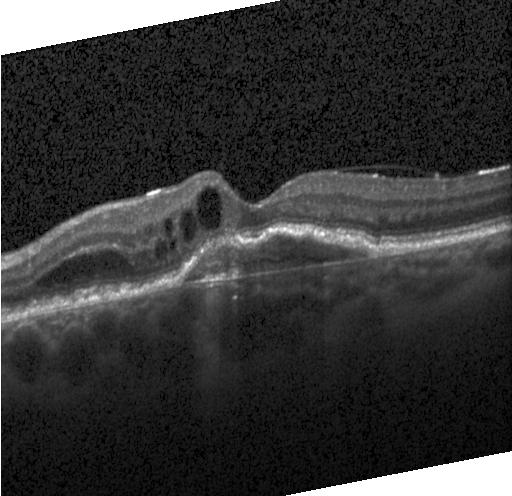 Impression: CNV.